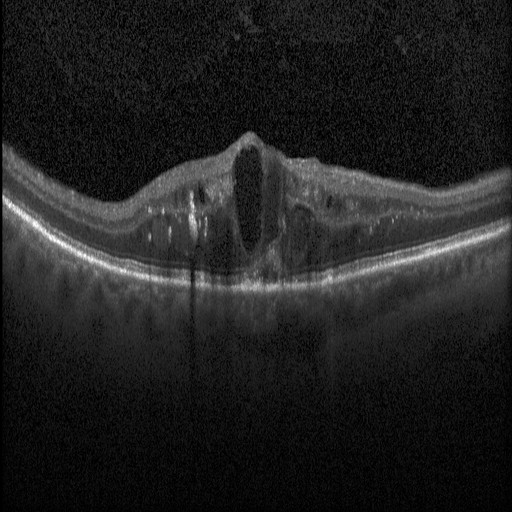
Spectral-domain optical coherence tomography · retinal OCT B-scan · instrument: Heidelberg Spectralis · horizontal scan through the fovea
DME.